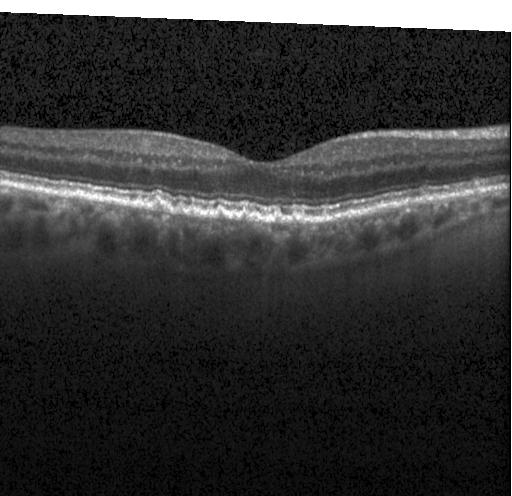
Diagnosis: drusen.